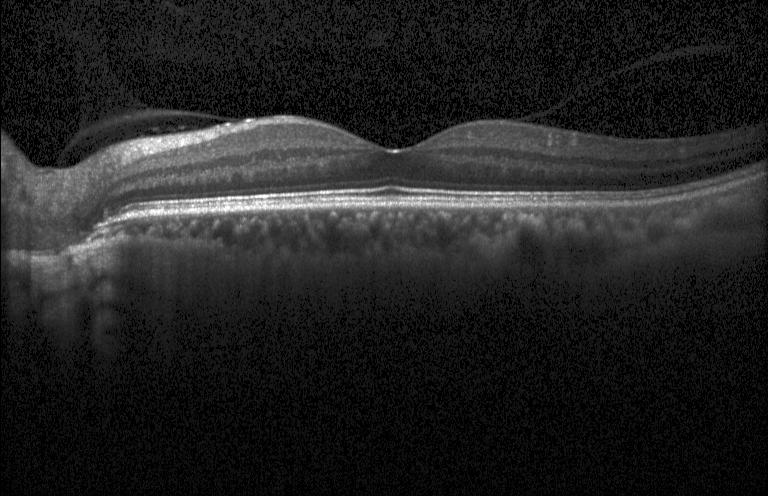

Centered on the fovea. Optical coherence tomography scan. Spectral-domain OCT. Macular OCT: no evidence of CNV, DME, or drusen.